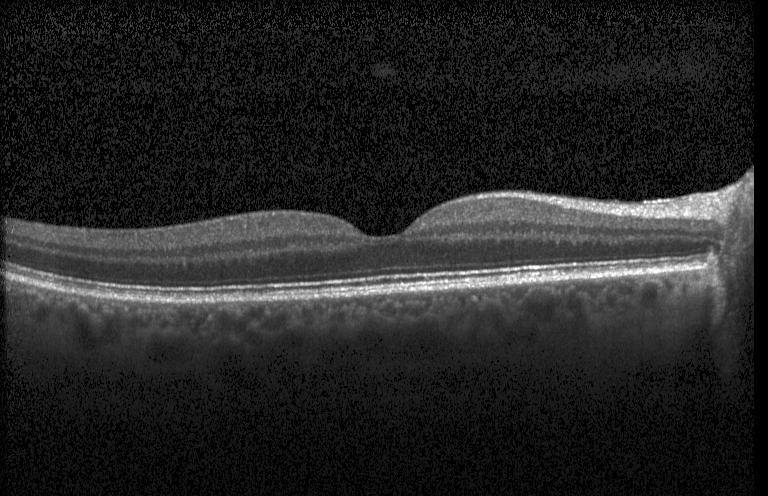 OCT B-scan · SD-OCT · through the macula. Diagnosis: neither CNV, DME, nor drusen.